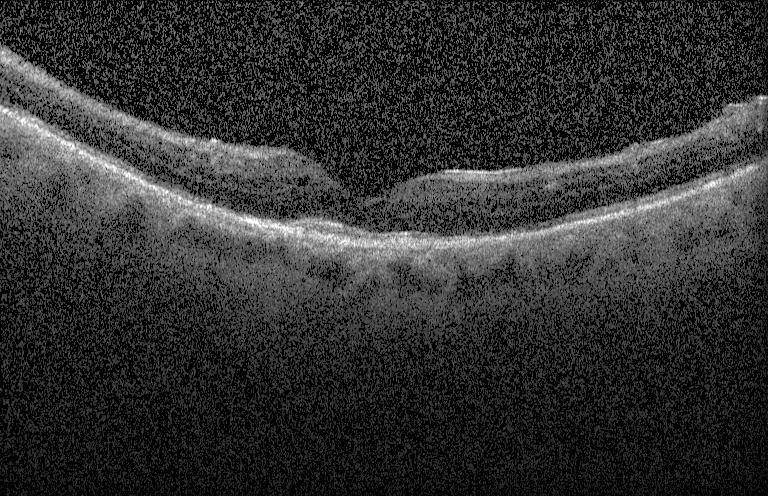

OCT B-scan — Choroidal neovascularization (CNV).